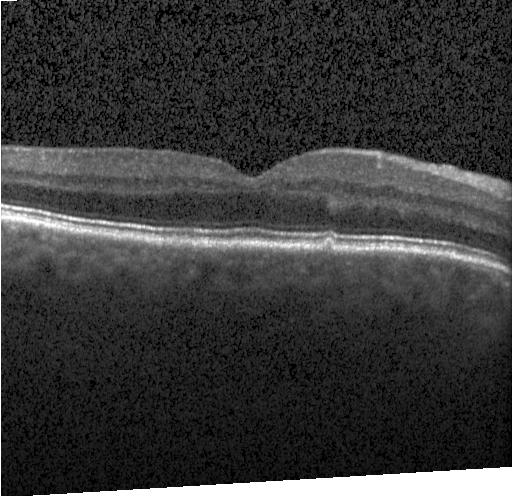 Assessment: sub-RPE drusenoid deposits.